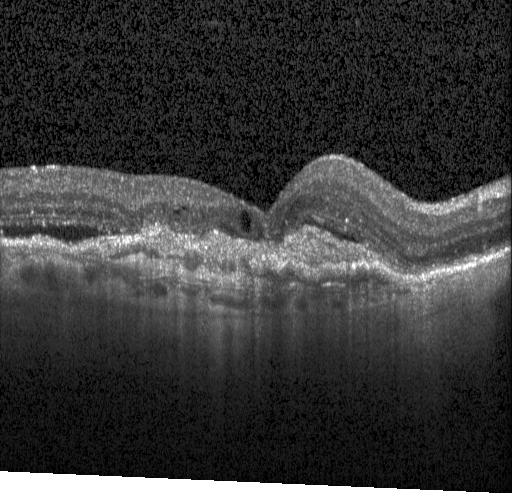 Diagnosis: CNV.